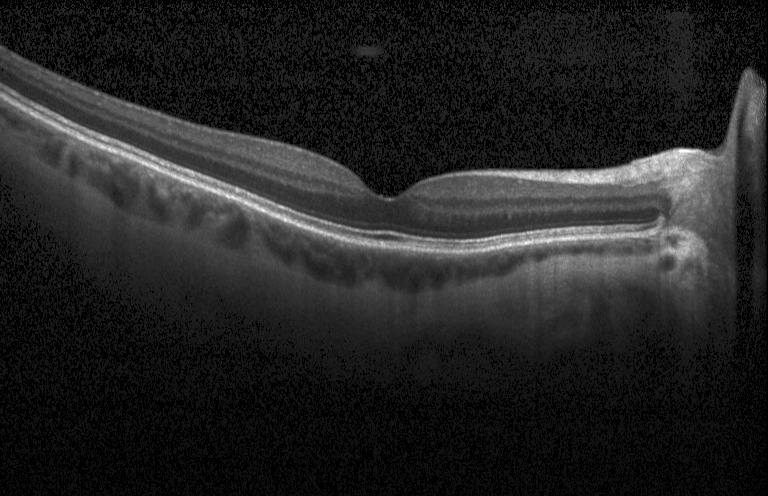
Retinal OCT cross-section — Dx: no evidence of choroidal neovascularization, diabetic macular edema, or drusen.